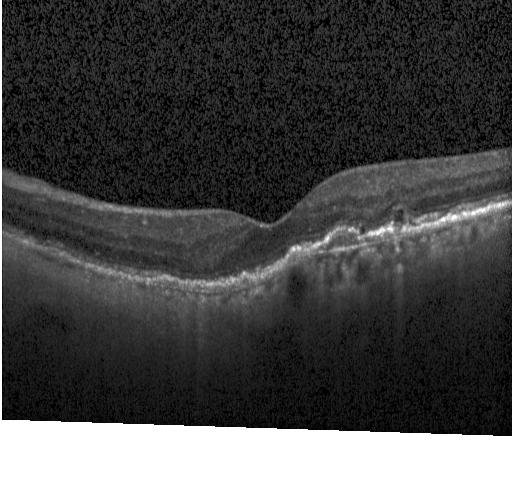 Centered on the fovea, optical coherence tomography B-scan, SD-OCT — Dx: a choroidal neovascular membrane.